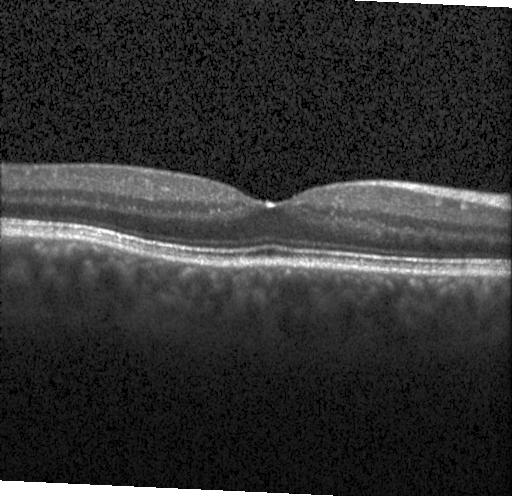
Retinal OCT cross-section — Macular OCT: no choroidal neovascularization, diabetic macular edema, or drusen.